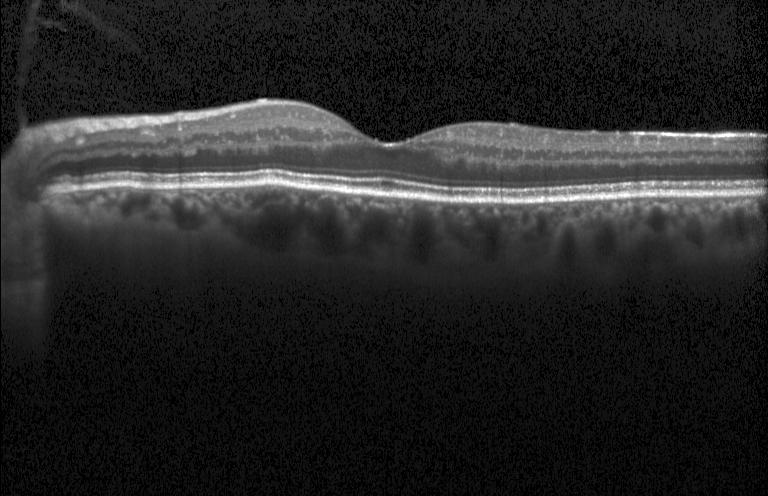 Horizontal scan through the fovea · spectral-domain OCT · OCT line scan. Impression: no evidence of choroidal neovascularization, diabetic macular edema, or drusen.